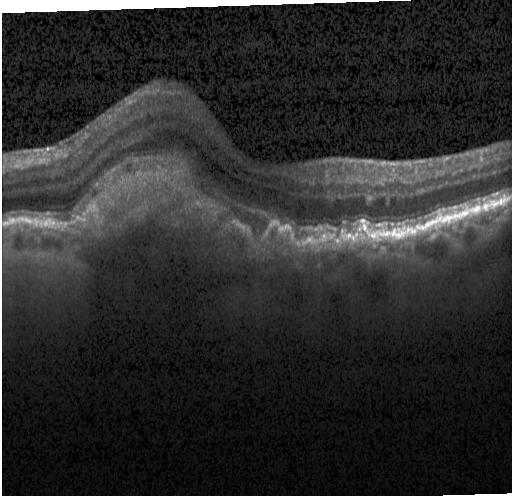

Retinal OCT cross-section; instrument: Heidelberg Spectralis. Finding: choroidal neovascularization.